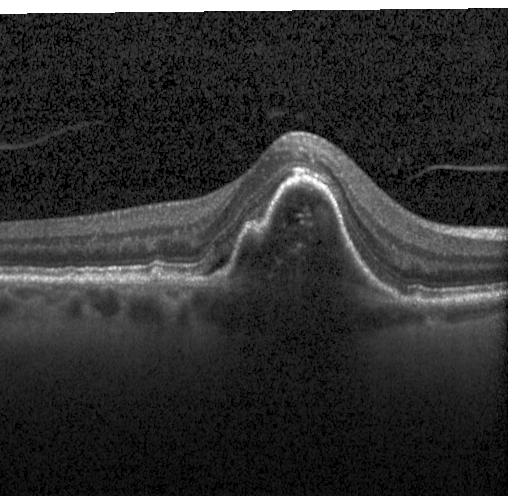 Optical coherence tomography B-scan. CNV.